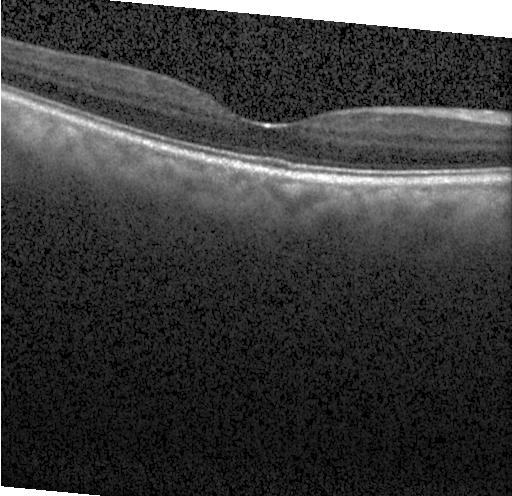
Impression: no evidence of choroidal neovascularization, diabetic macular edema, or drusen.